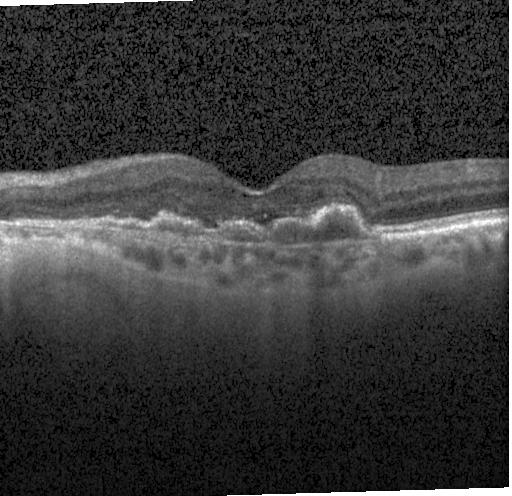
Finding: CNV.